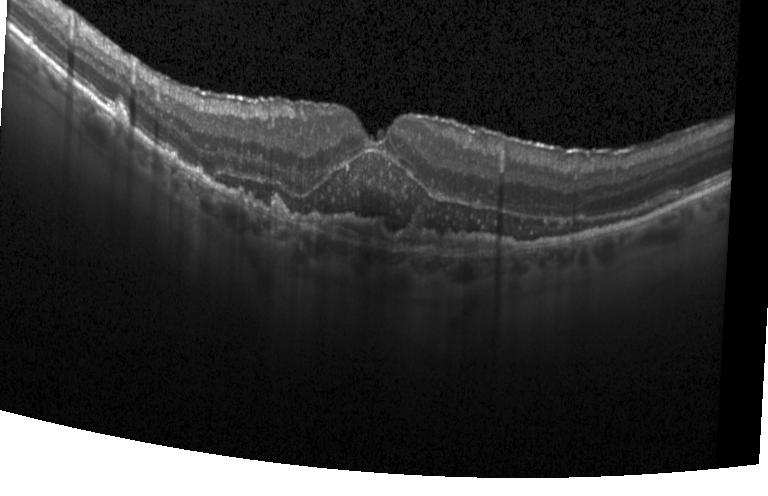

SD-OCT; centered on the fovea; retinal OCT B-scan; Heidelberg Spectralis OCT system — Impression: a choroidal neovascular membrane.